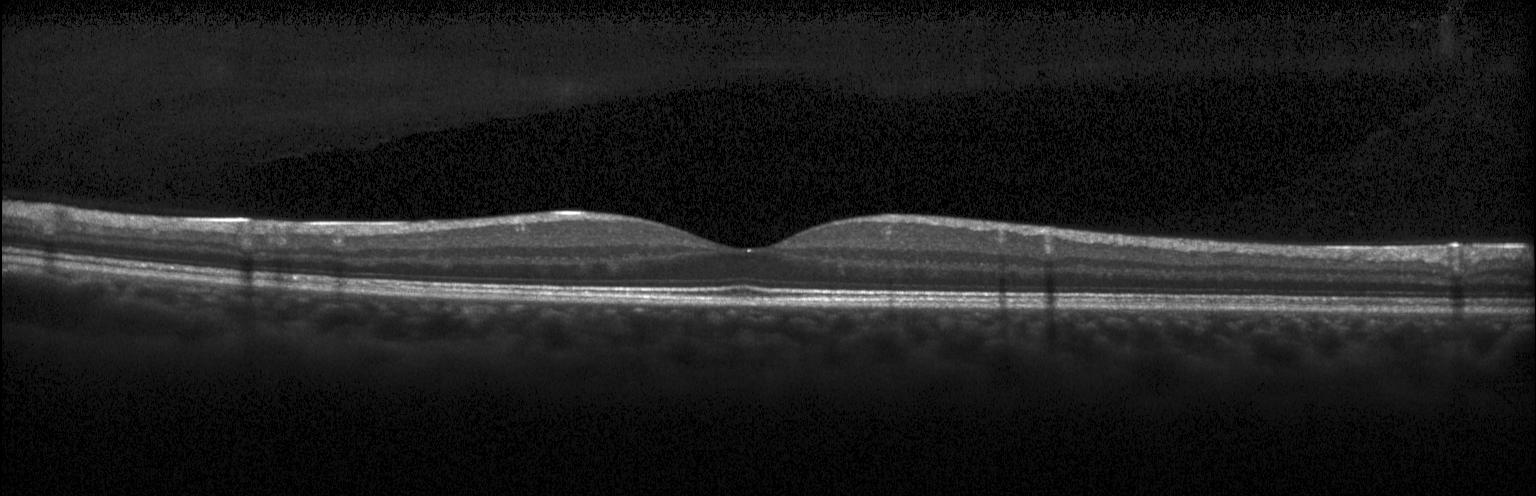

Retinal OCT B-scan, acquired on a Heidelberg Spectralis
The scan shows no choroidal neovascularization, diabetic macular edema, or drusen.